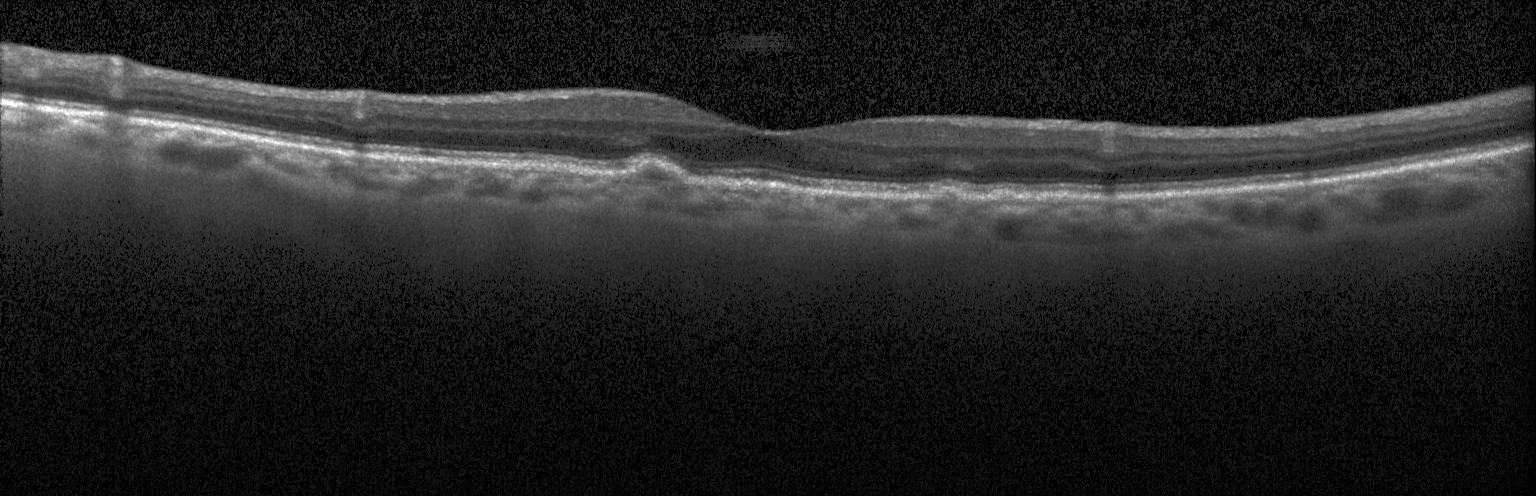 Impression: drusen.